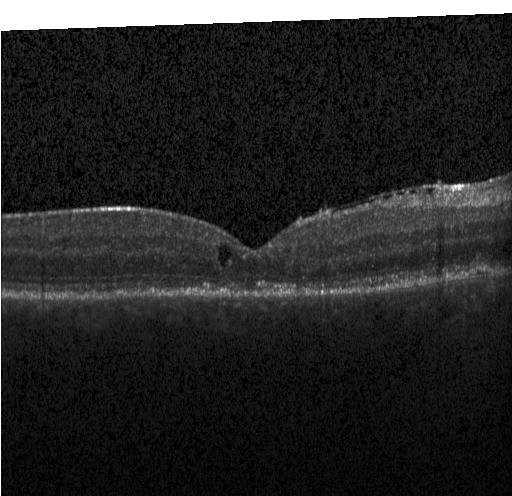
Spectral-domain optical coherence tomography; retinal OCT cross-section — Impression: diabetic macular edema.